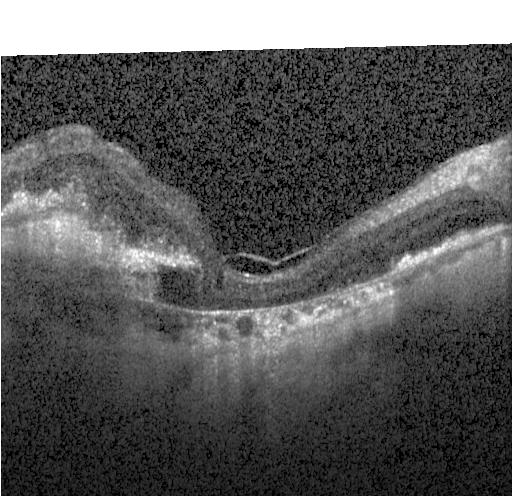

A choroidal neovascular membrane.